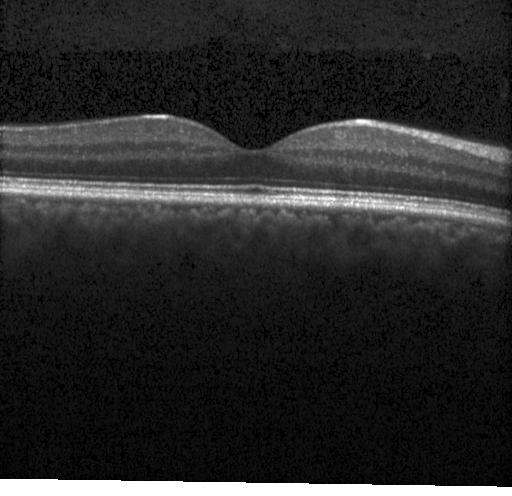
Optical coherence tomography B-scan.
Impression: no CNV, DME, or drusen.